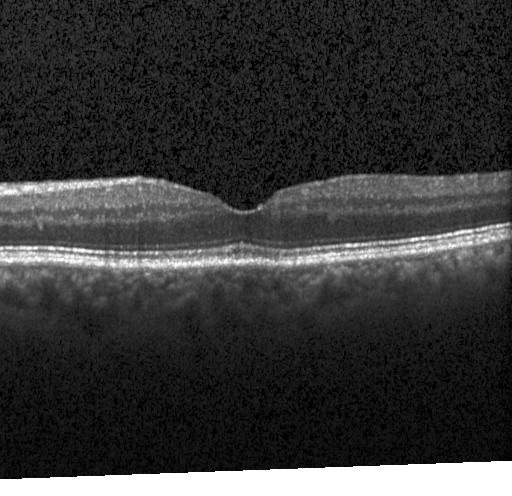

Finding: no evidence of choroidal neovascularization, diabetic macular edema, or drusen.